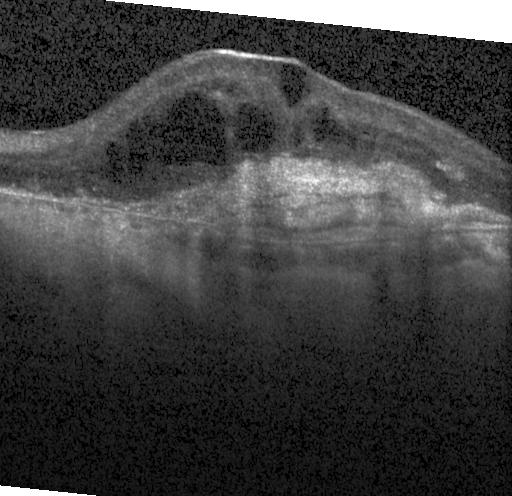
Retinal OCT B-scan — A choroidal neovascular membrane.